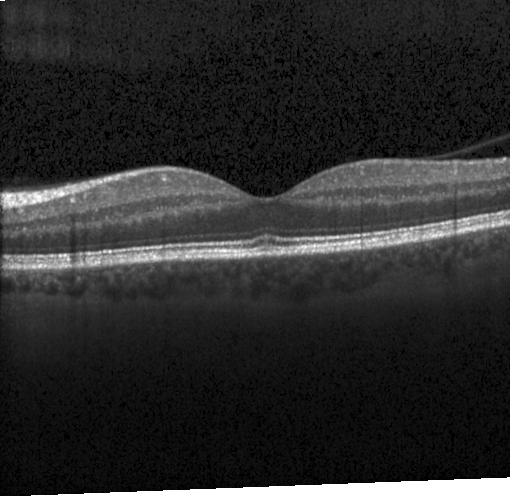
This B-scan demonstrates no CNV, no DME, and no drusen.